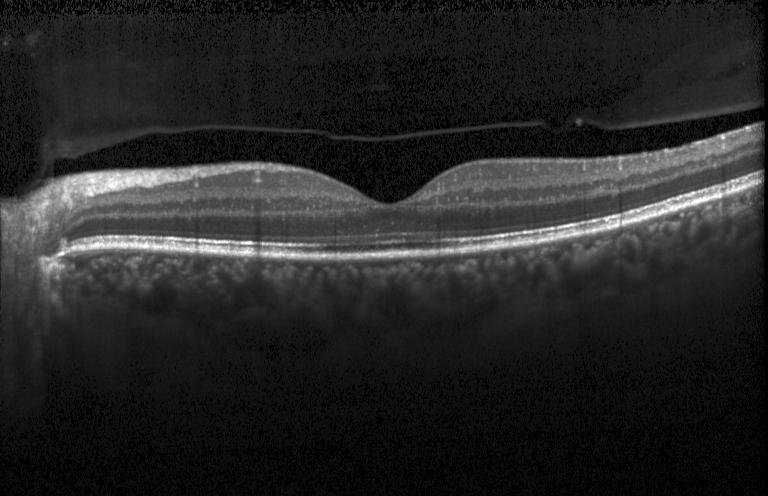
Diagnosis: no evidence of CNV, DME, or drusen.